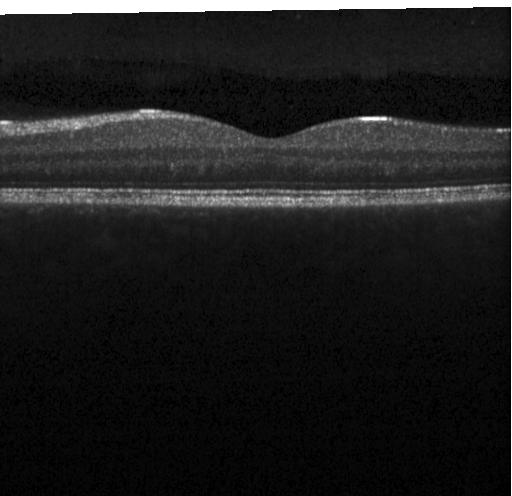
SD-OCT. OCT line scan — Impression: no choroidal neovascularization, no diabetic macular edema, and no drusen.